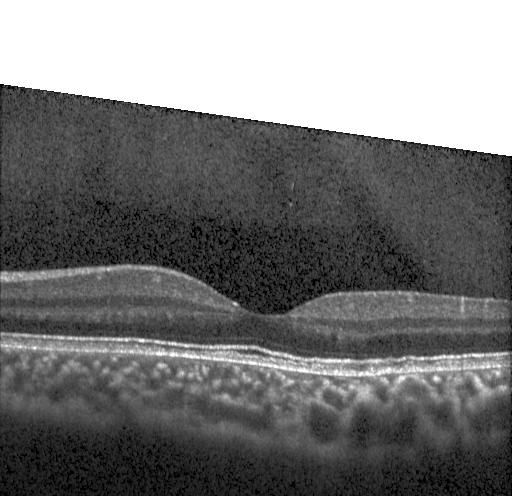
Optical coherence tomography scan. Spectral-domain optical coherence tomography. Diagnosis: no choroidal neovascularization, diabetic macular edema, or drusen.